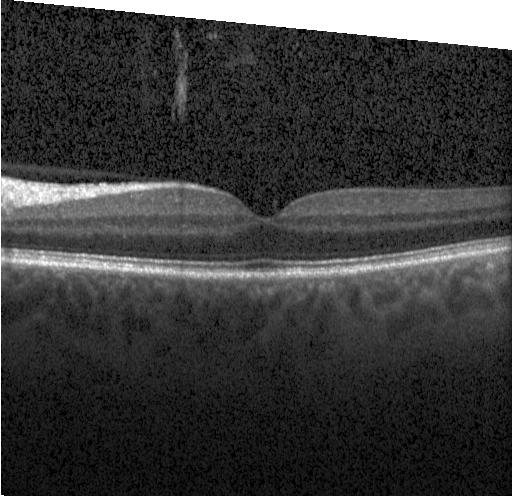
Finding: no CNV, DME, or drusen.